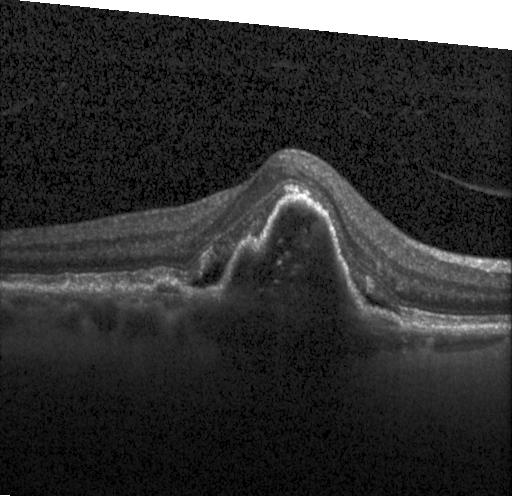

Instrument: Heidelberg Spectralis · OCT line scan
Diagnosis: a choroidal neovascular membrane.